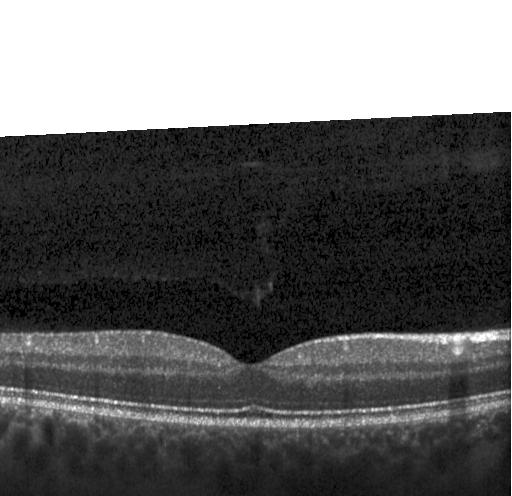

Spectral-domain OCT B-scan: no CNV, no DME, and no drusen.